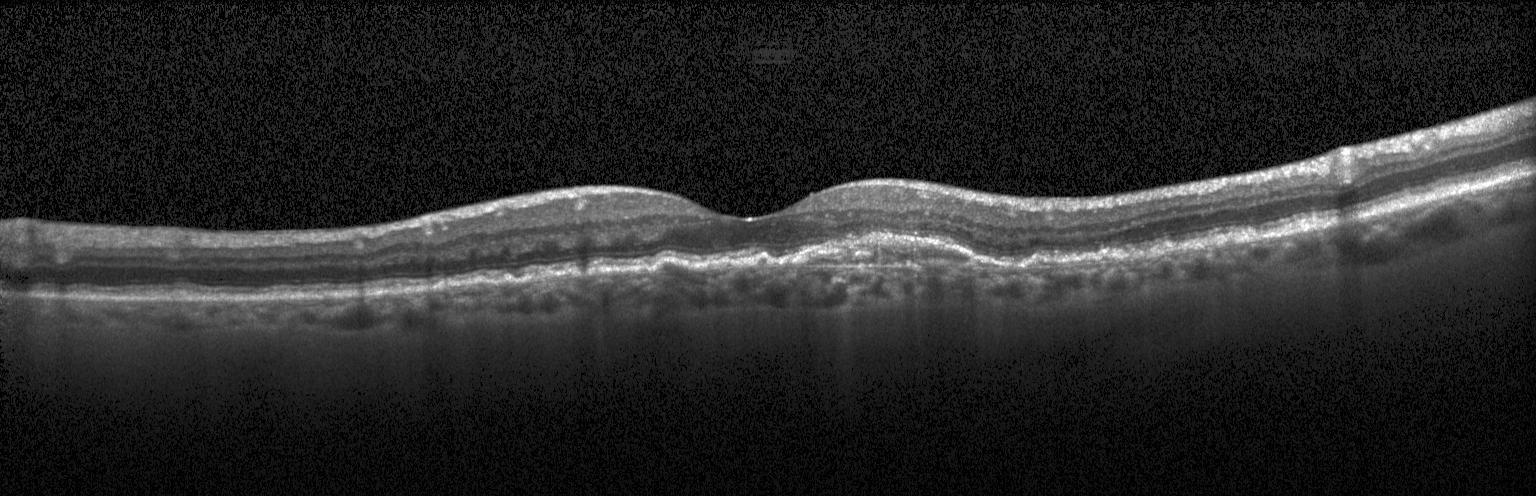

Macular scan, spectral-domain optical coherence tomography, optical coherence tomography B-scan. Impression: choroidal neovascularization.